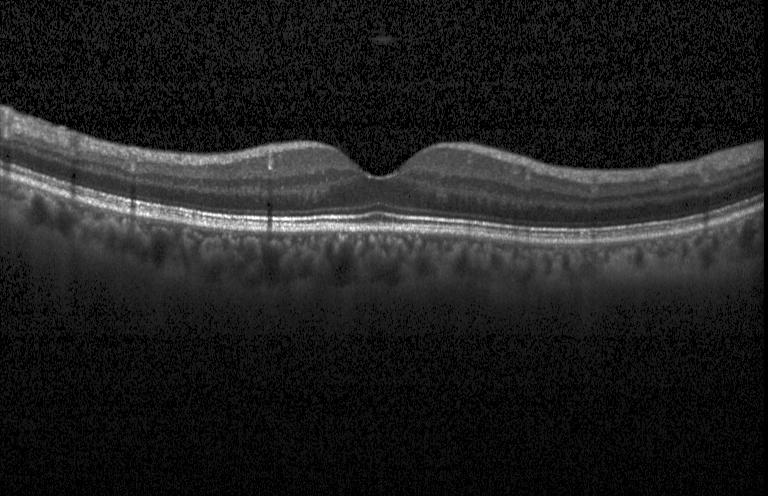
Retinal OCT cross-section — This B-scan demonstrates neither choroidal neovascularization, diabetic macular edema, nor drusen.